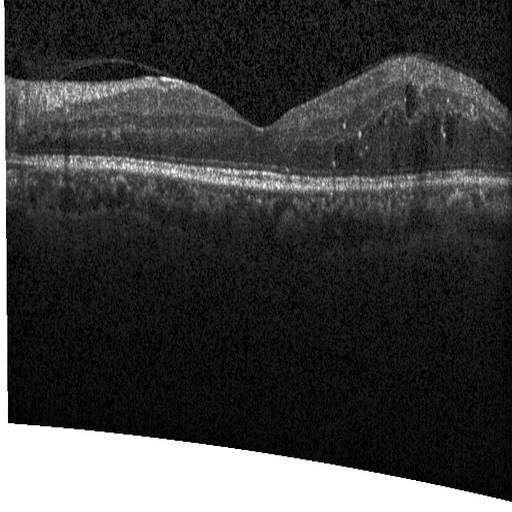

Fovea-centered, spectral-domain OCT, retinal OCT cross-section — Impression: diabetic macular edema (DME).